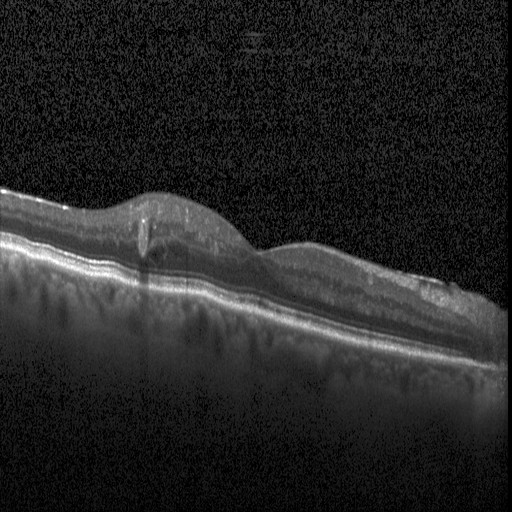 Diagnosis: diabetic macular edema (DME).